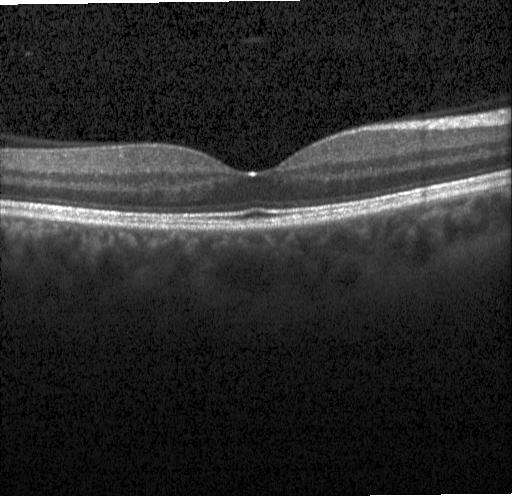 OCT B-scan, Heidelberg Spectralis, spectral-domain OCT
This B-scan demonstrates no evidence of choroidal neovascularization, diabetic macular edema, or drusen.